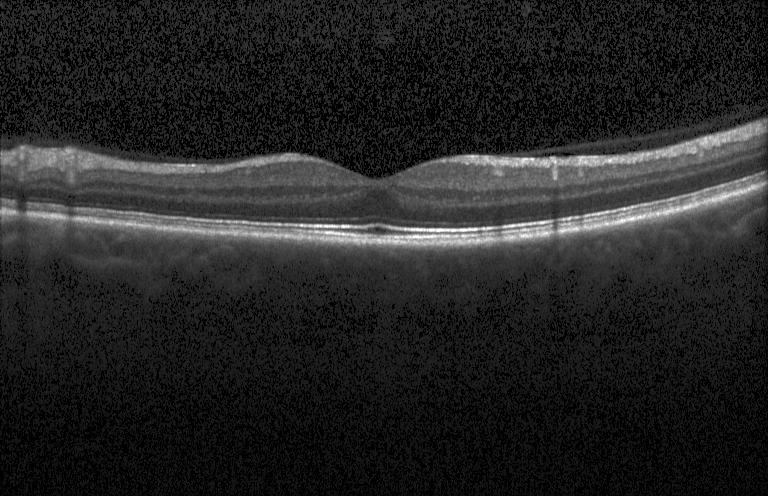

Retinal OCT cross-section
Finding: neither choroidal neovascularization, diabetic macular edema, nor drusen.